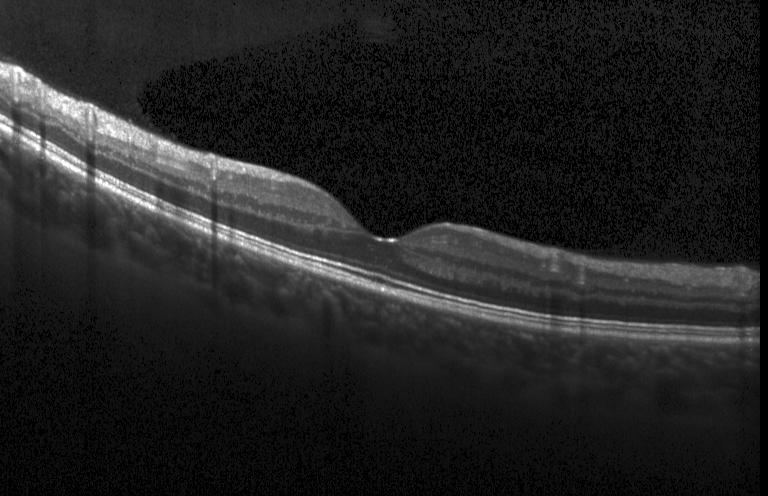 No evidence of choroidal neovascularization, diabetic macular edema, or drusen.